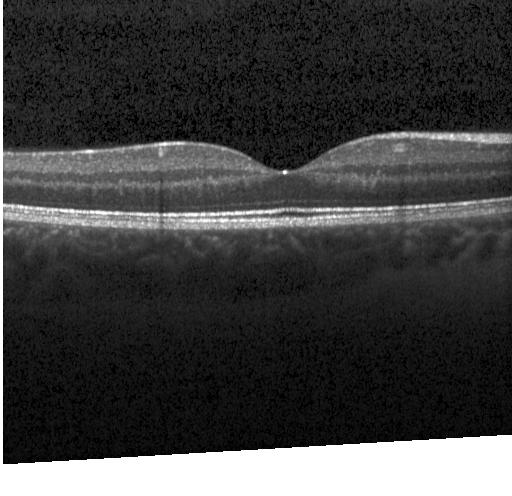 OCT line scan
Assessment: no CNV, no DME, and no drusen.